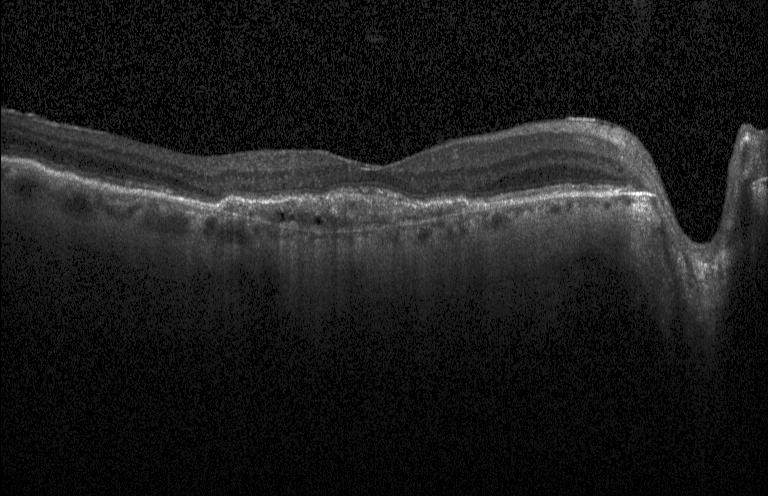 Retinal OCT B-scan.
Diagnosis: choroidal neovascularization.